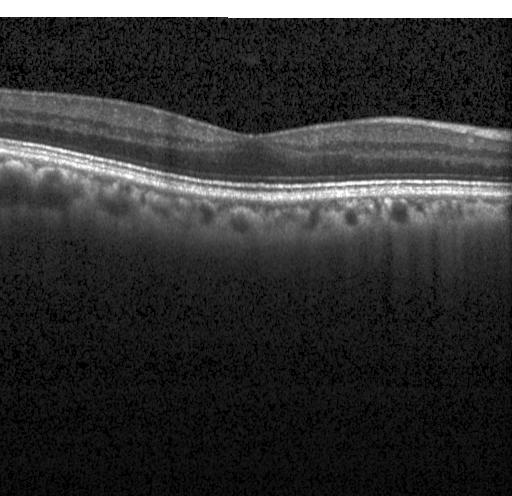

Acquired on a Heidelberg Spectralis; spectral-domain optical coherence tomography; through the macula; retinal OCT cross-section — OCT finding: no evidence of choroidal neovascularization, diabetic macular edema, or drusen.